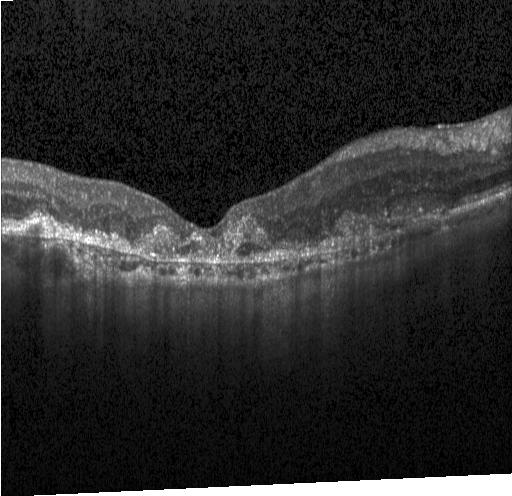
Spectral-domain OCT B-scan: a choroidal neovascular membrane.